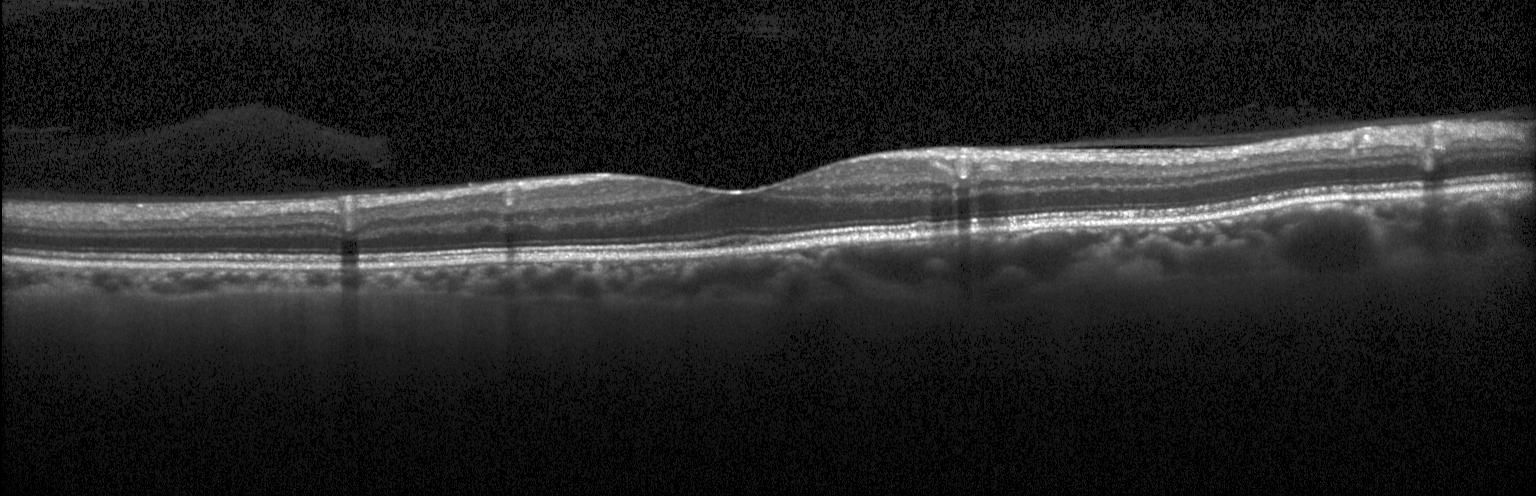

Macular OCT: no evidence of CNV, DME, or drusen.